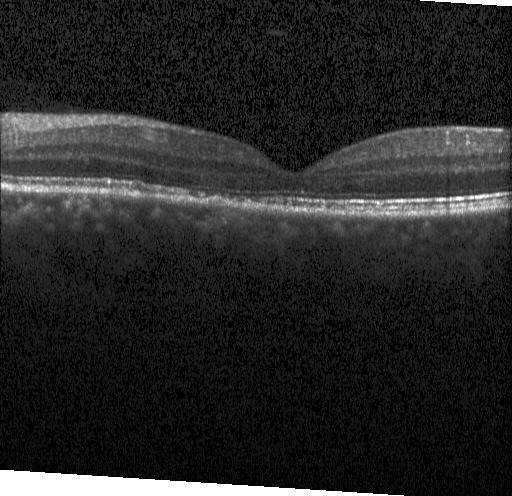
Through the macula, SD-OCT, OCT line scan
This B-scan demonstrates no evidence of choroidal neovascularization, diabetic macular edema, or drusen.